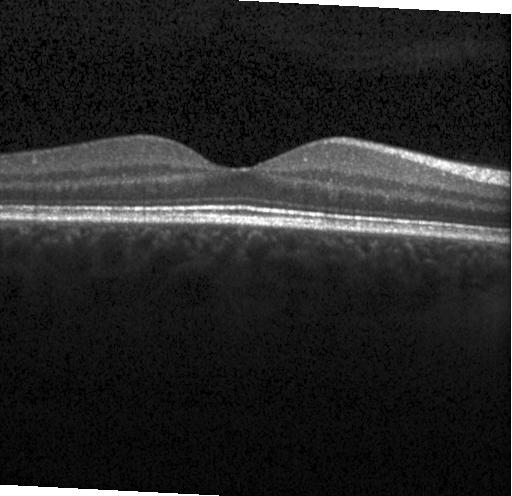
OCT B-scan; macular scan; Heidelberg Spectralis.
Finding: no choroidal neovascularization, no diabetic macular edema, and no drusen.